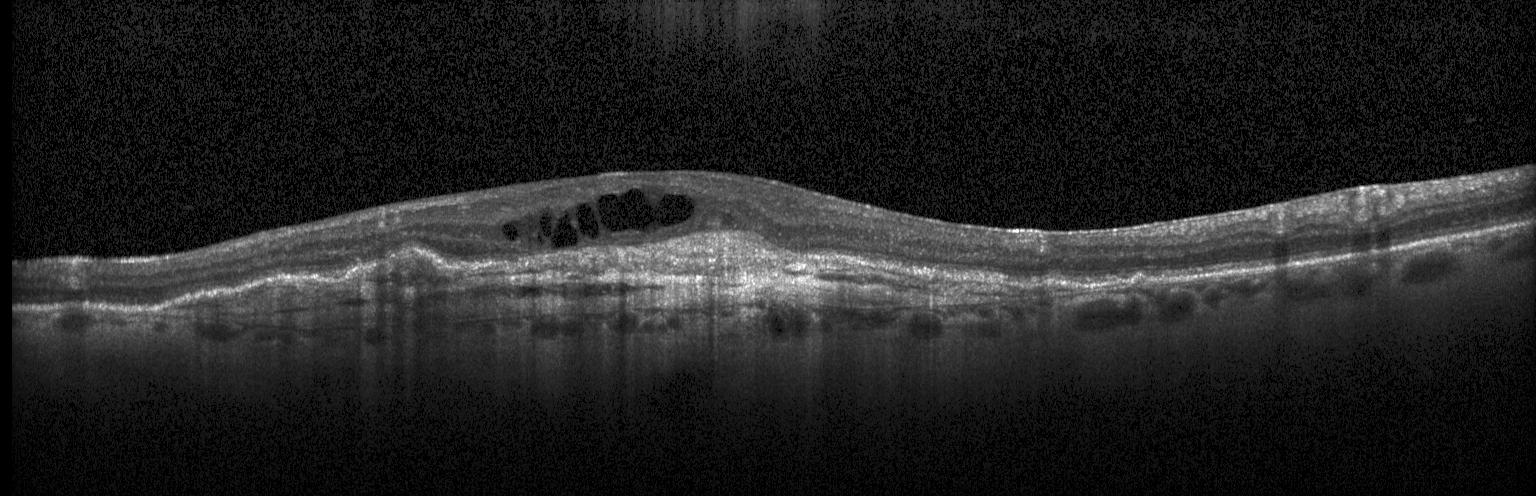 Centered on the fovea. OCT line scan. SD-OCT. Heidelberg Spectralis OCT system
OCT finding: a choroidal neovascular membrane.